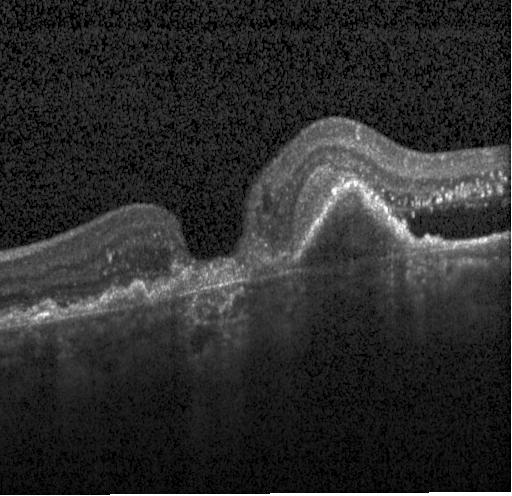

Diagnosis: choroidal neovascularization.